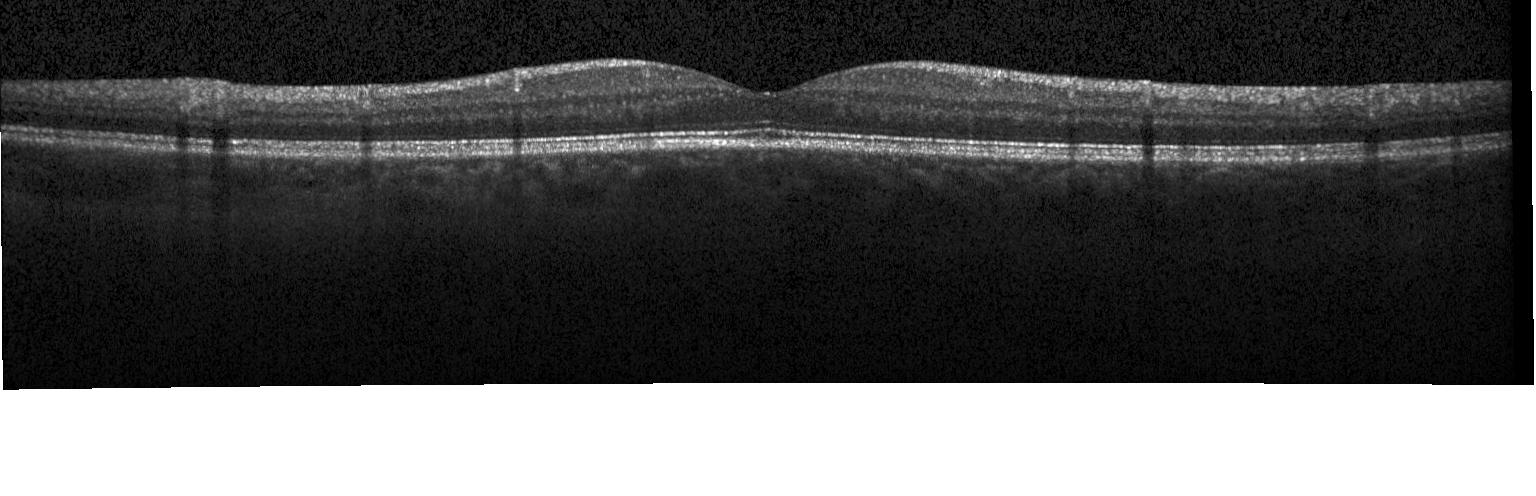 Optical coherence tomography scan, spectral-domain optical coherence tomography — Diagnosis: neither choroidal neovascularization, diabetic macular edema, nor drusen.